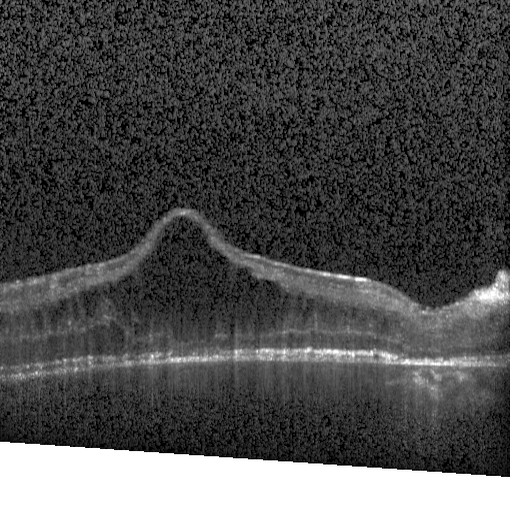 Optical coherence tomography scan.
Finding: DME.